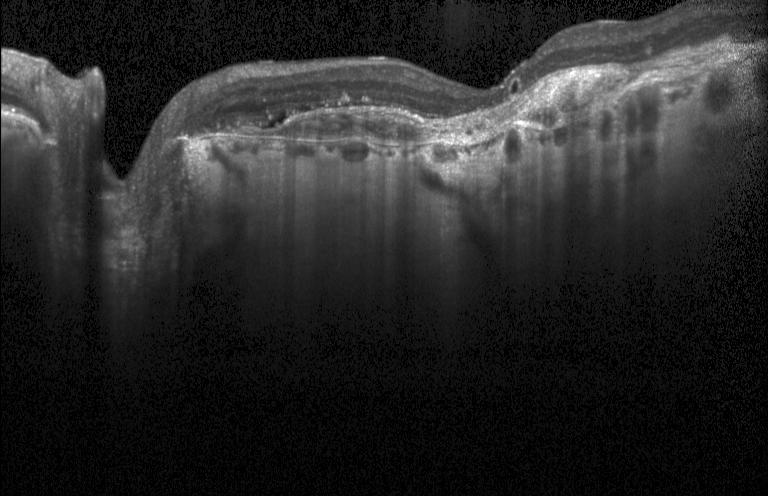
Dx: a choroidal neovascular membrane.